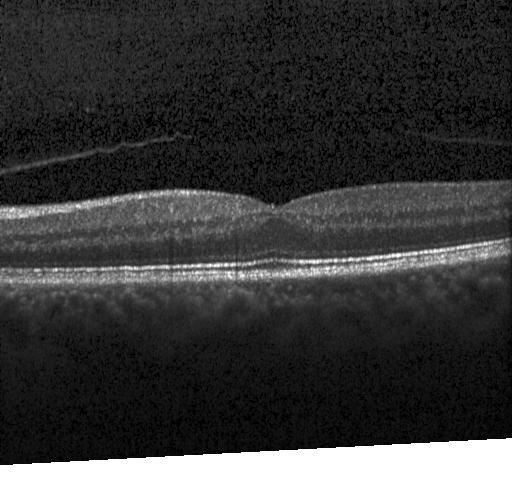
OCT line scan.
Diagnosis: neither CNV, DME, nor drusen.